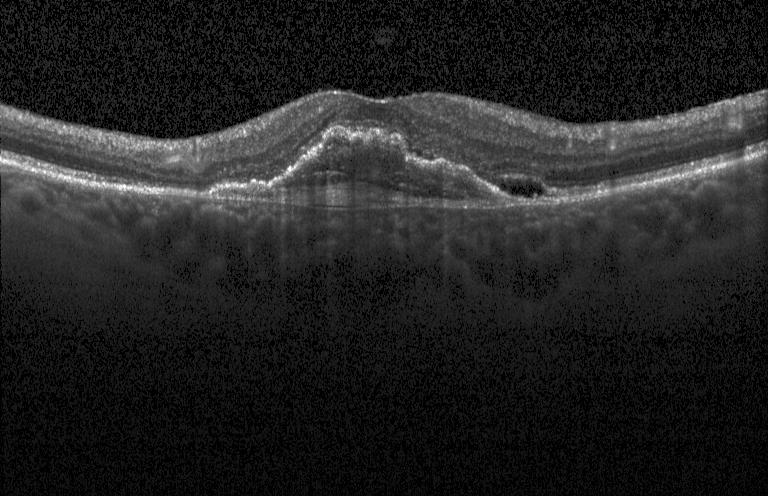

Through the macula, spectral-domain OCT, instrument: Heidelberg Spectralis, retinal OCT B-scan. Impression: a choroidal neovascular membrane.